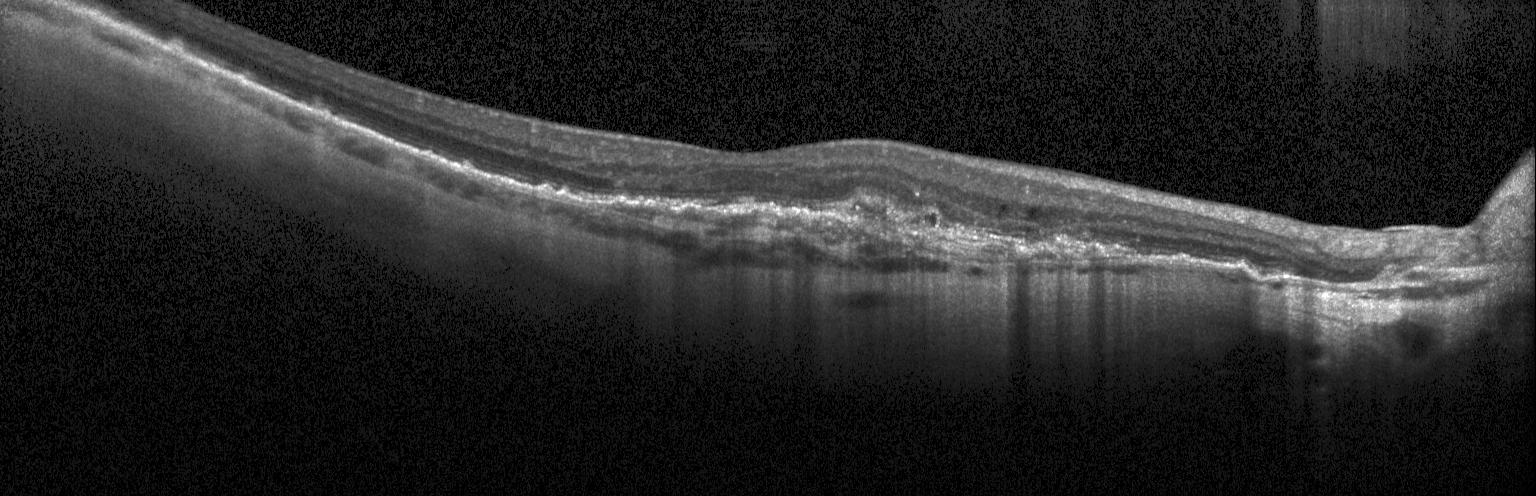

Retinal OCT cross-section.
Macular OCT: a choroidal neovascular membrane.